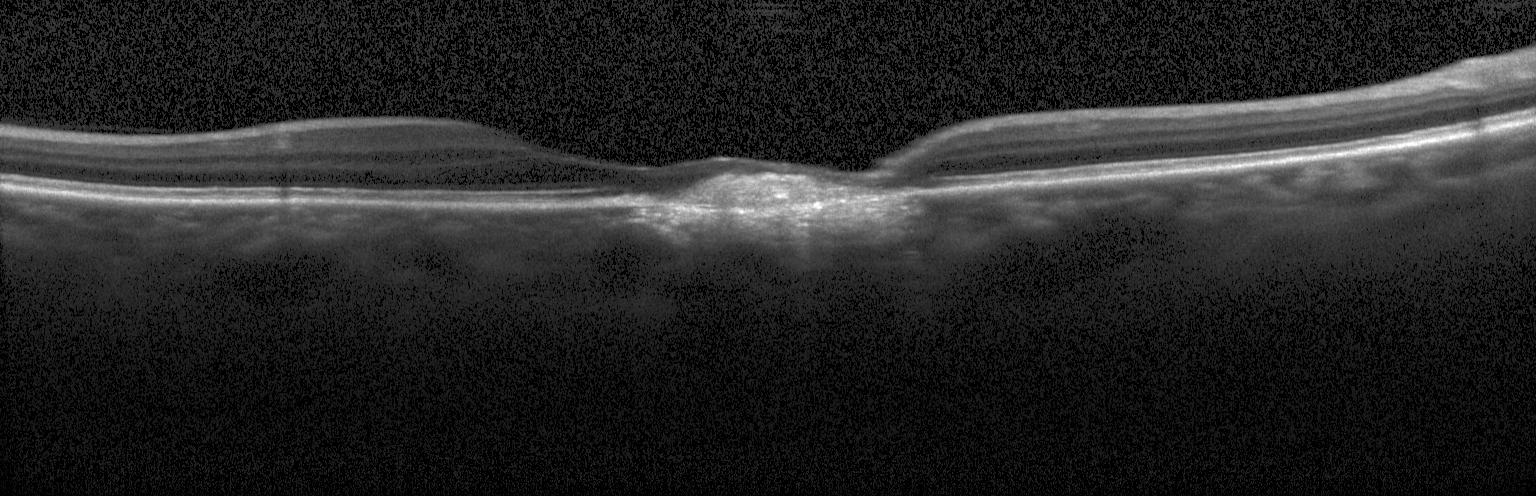 Macular scan · retinal OCT cross-section — The scan shows a choroidal neovascular membrane.